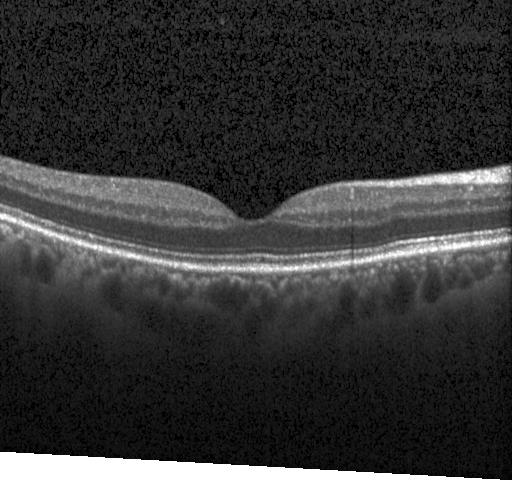 Retinal OCT cross-section, through the macula.
Impression: no choroidal neovascularization, diabetic macular edema, or drusen.